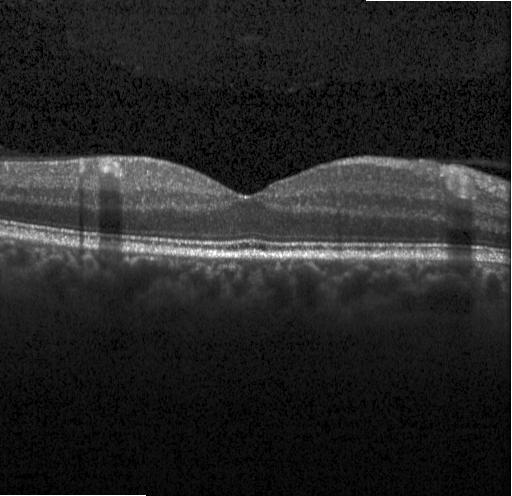
Optical coherence tomography scan. Finding: no CNV, DME, or drusen.